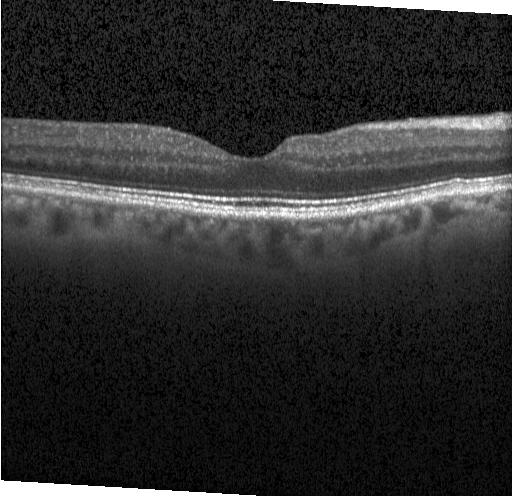
Heidelberg Spectralis OCT system. Spectral-domain optical coherence tomography. OCT line scan. Finding: neither CNV, DME, nor drusen.